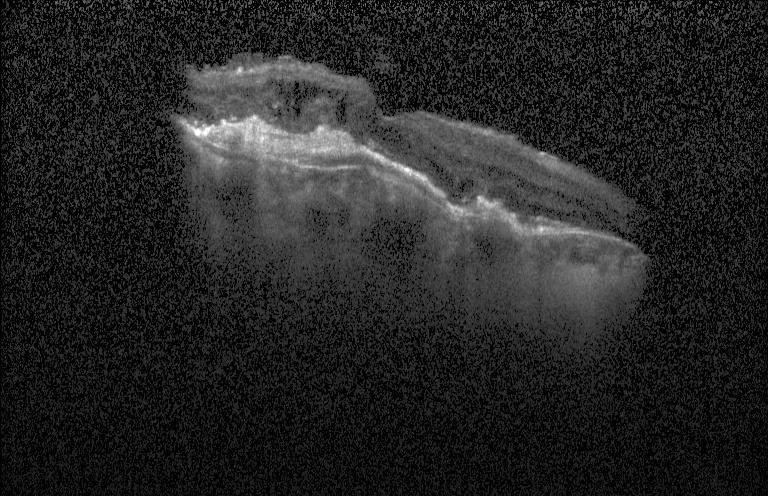

CNV.